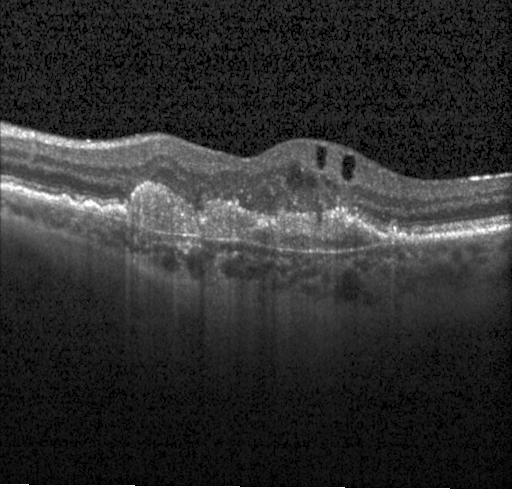 Through the macula, optical coherence tomography B-scan, acquired on a Heidelberg Spectralis, SD-OCT — Impression: CNV.